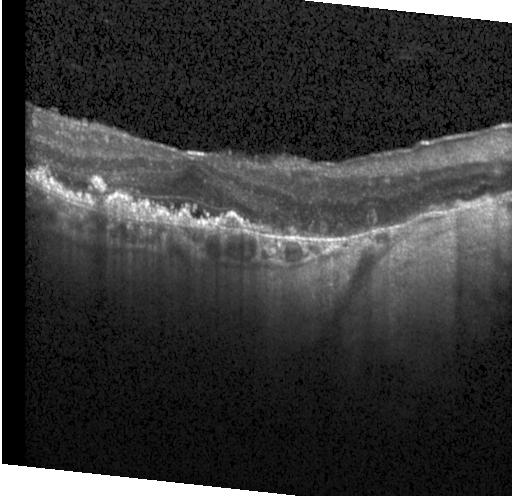
Optical coherence tomography scan, Heidelberg Spectralis, macular scan, SD-OCT. Dx: CNV.